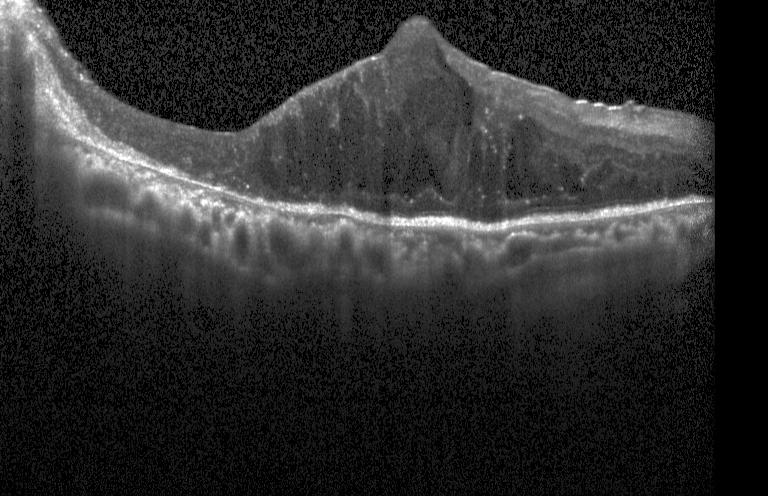

Retinal OCT cross-section, acquired on a Heidelberg Spectralis
Finding: DME.